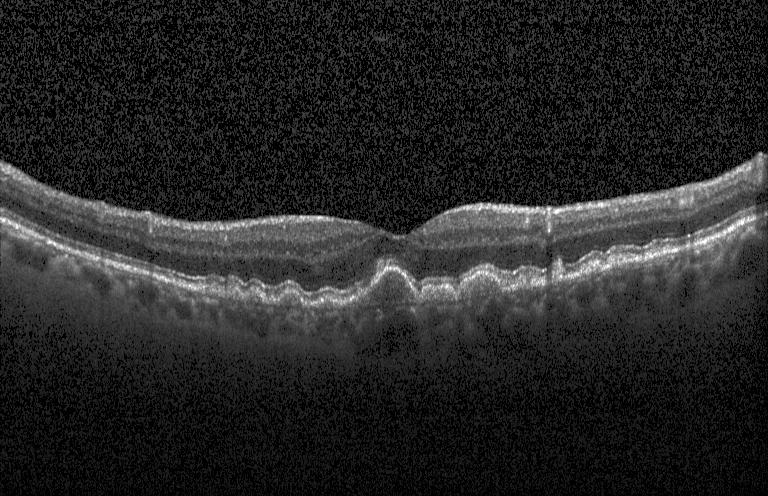

Finding: multiple drusen.